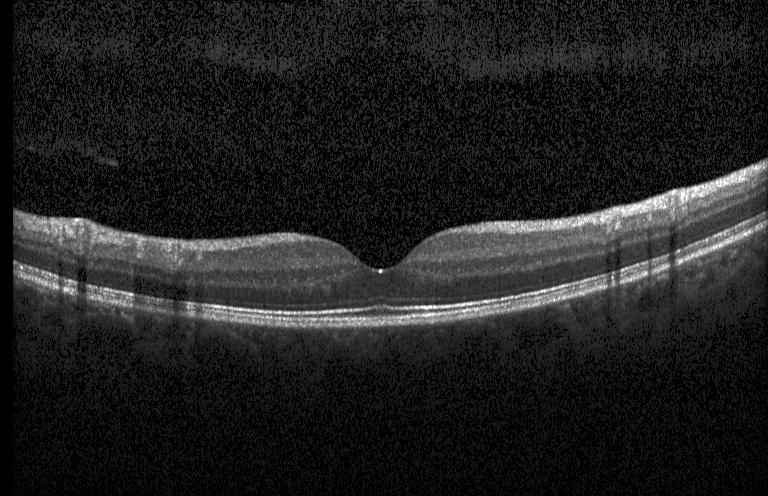
Heidelberg Spectralis, optical coherence tomography B-scan.
Diagnosis: no evidence of choroidal neovascularization, diabetic macular edema, or drusen.